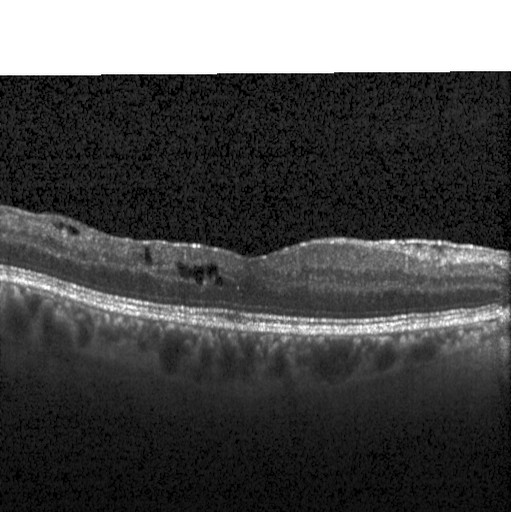 Retinal OCT cross-section showing diabetic macular edema (DME).